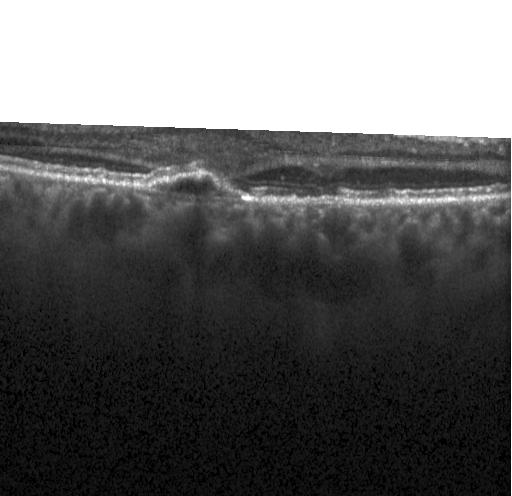 OCT line scan
This B-scan demonstrates choroidal neovascularization.